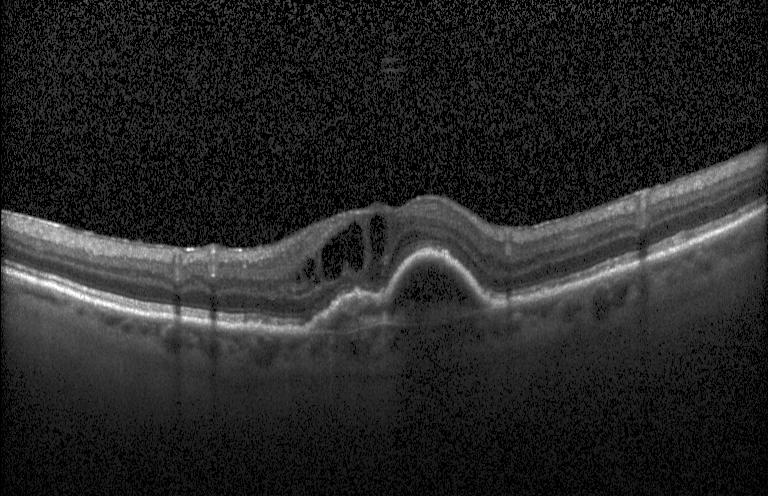 Retinal OCT B-scan.
The scan shows choroidal neovascularization.